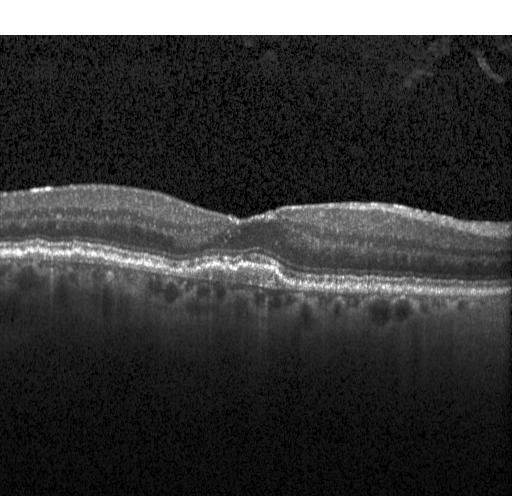 OCT B-scan showing a choroidal neovascular membrane.